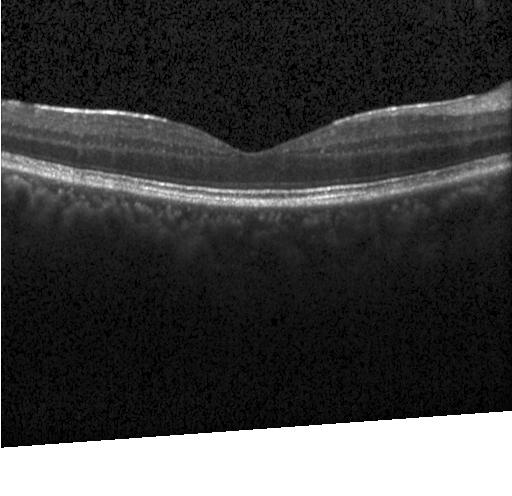

This B-scan demonstrates no choroidal neovascularization, no diabetic macular edema, and no drusen.